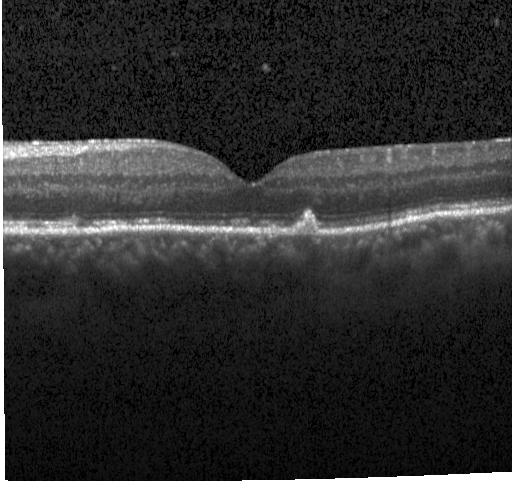

Dx: sub-RPE drusenoid deposits.